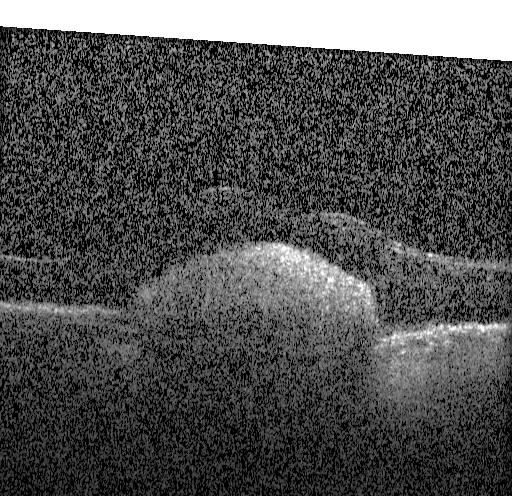
Retinal OCT cross-section.
Dx: choroidal neovascularization (CNV).